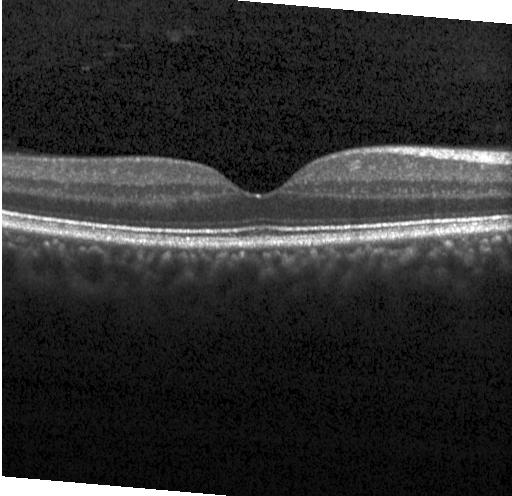 Retinal OCT B-scan — Finding: no evidence of choroidal neovascularization, diabetic macular edema, or drusen.